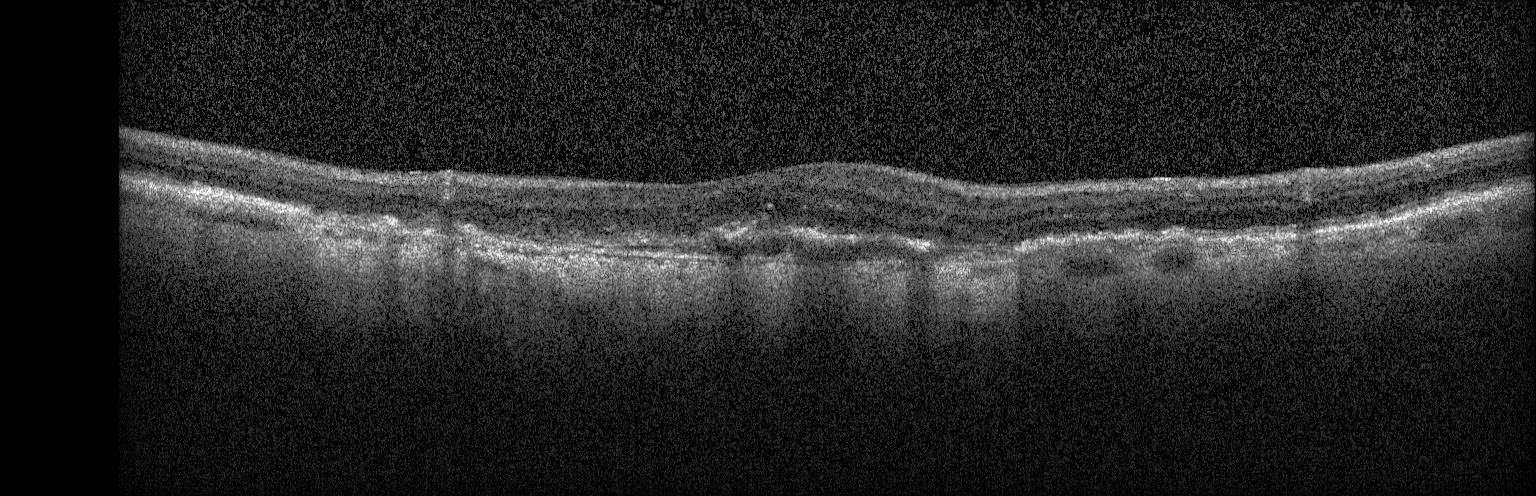
Heidelberg Spectralis, retinal OCT cross-section, fovea-centered — Assessment: a choroidal neovascular membrane.